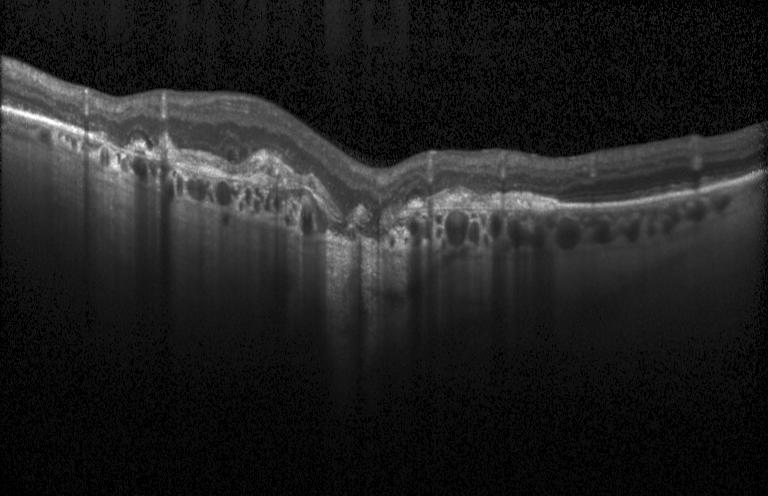

Retinal OCT B-scan, spectral-domain OCT, acquired on a Heidelberg Spectralis, macular scan — CNV.